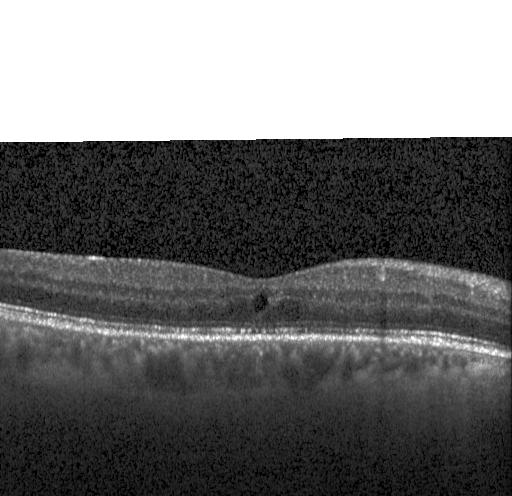 Finding: diabetic macular edema.